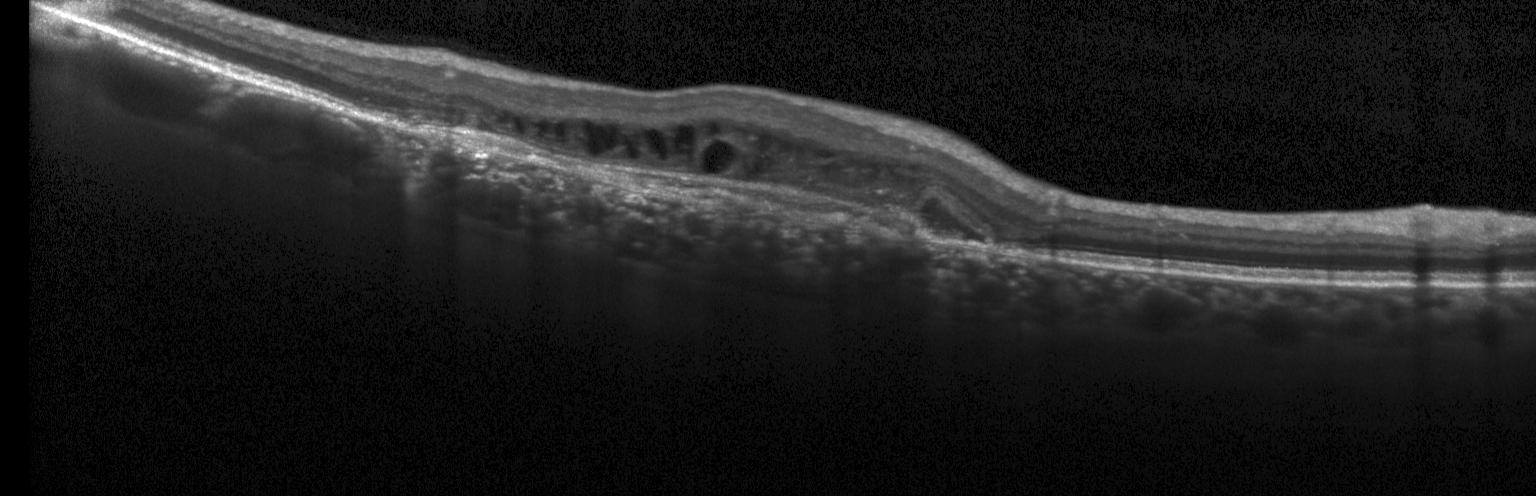
Spectral-domain OCT · retinal OCT B-scan · macular scan — Dx: a choroidal neovascular membrane.